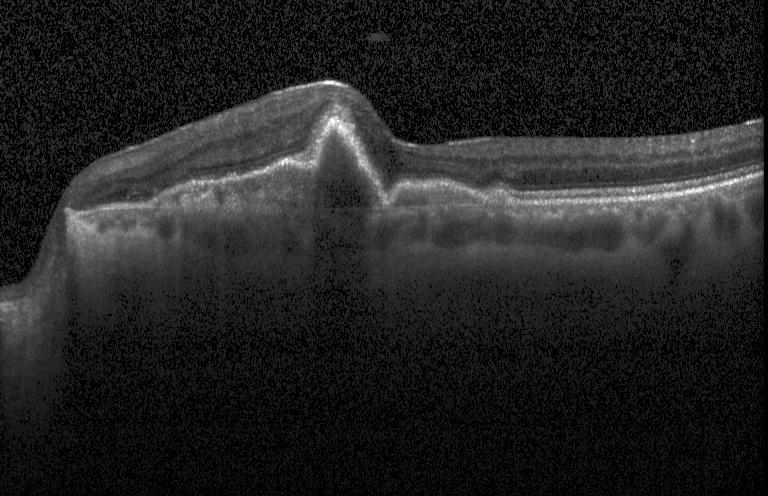

Macular OCT: a choroidal neovascular membrane.